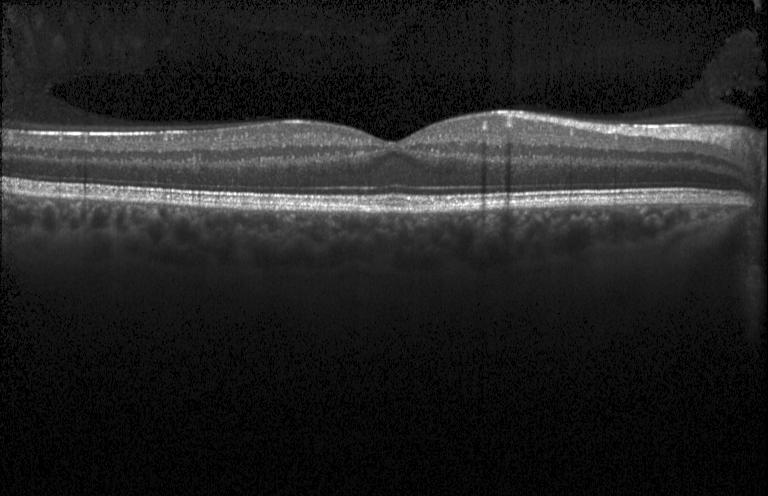
Optical coherence tomography scan, spectral-domain optical coherence tomography, macular scan.
This B-scan demonstrates neither choroidal neovascularization, diabetic macular edema, nor drusen.